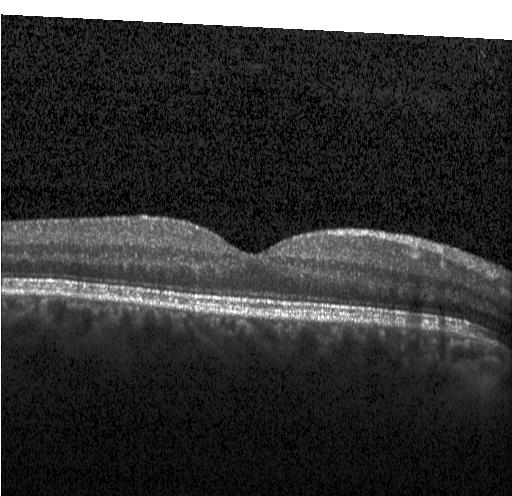

Horizontal scan through the fovea. Heidelberg Spectralis. Retinal OCT B-scan. Spectral-domain optical coherence tomography. No evidence of choroidal neovascularization, diabetic macular edema, or drusen.